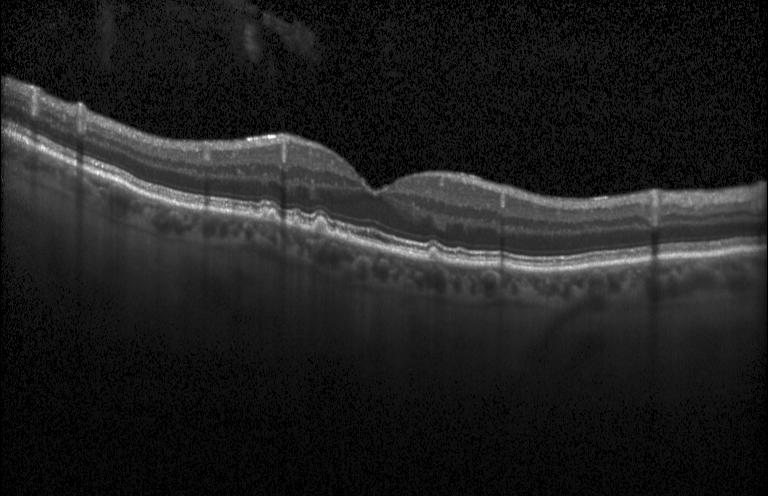

OCT B-scan.
Finding: multiple drusen.